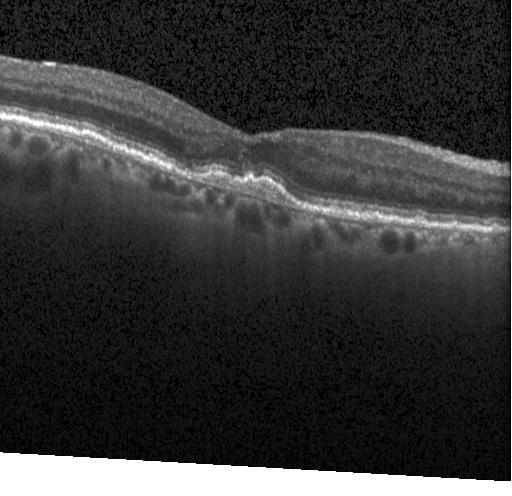
Spectral-domain OCT; retinal OCT B-scan; Heidelberg Spectralis OCT system. Impression: a choroidal neovascular membrane.